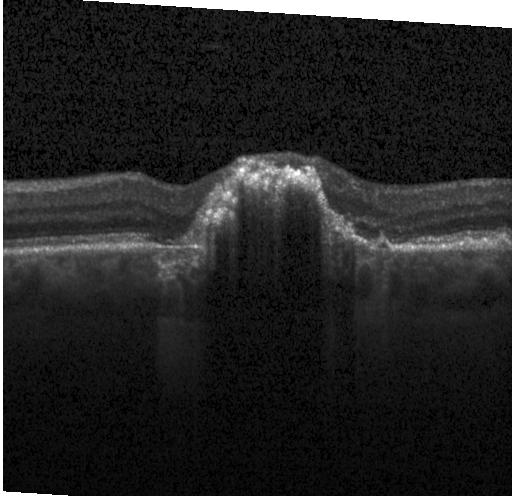 OCT B-scan, Heidelberg Spectralis OCT system, spectral-domain optical coherence tomography
Diagnosis: CNV.